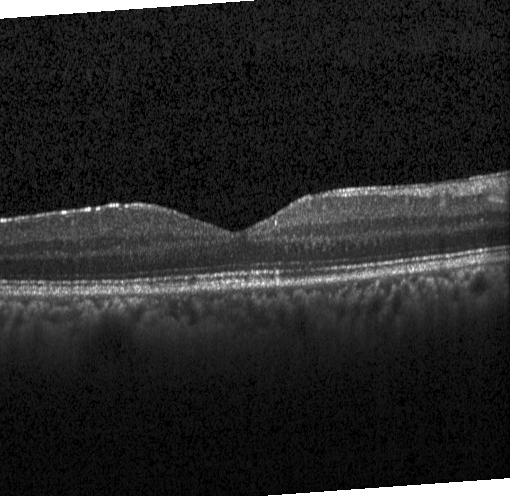 Retinal OCT B-scan, SD-OCT, Heidelberg Spectralis OCT system, horizontal scan through the fovea — Finding: no CNV, no DME, and no drusen.